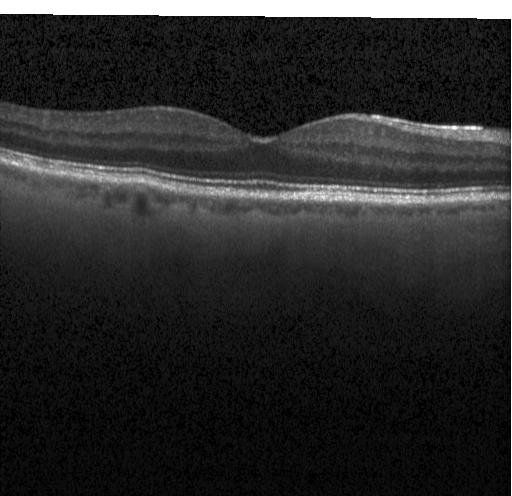 OCT line scan. The scan shows no CNV, DME, or drusen.